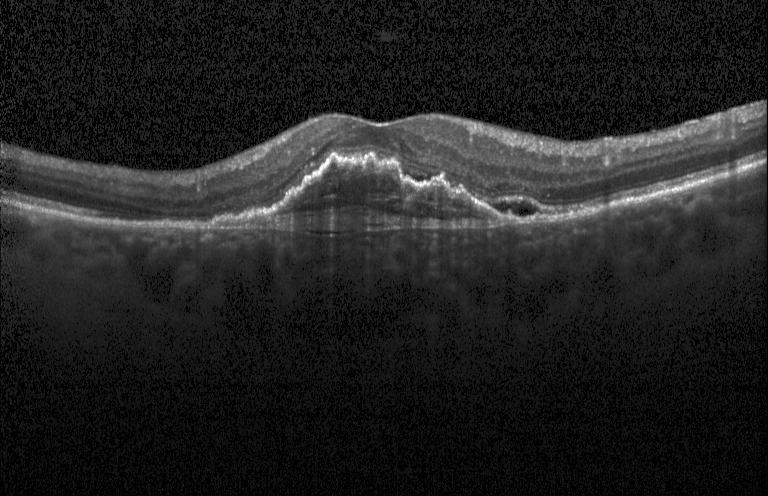 Retinal OCT cross-section. This B-scan demonstrates a choroidal neovascular membrane.